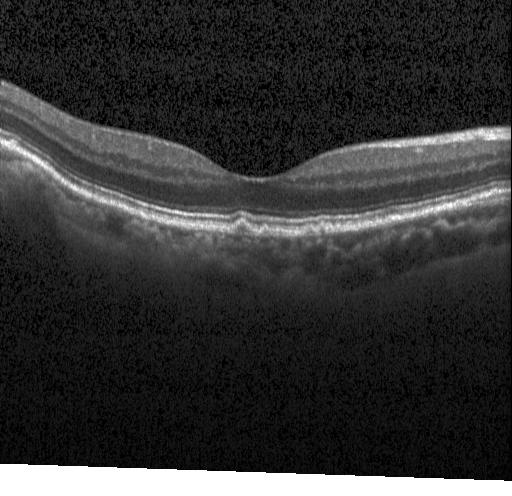

OCT scan showing drusen.